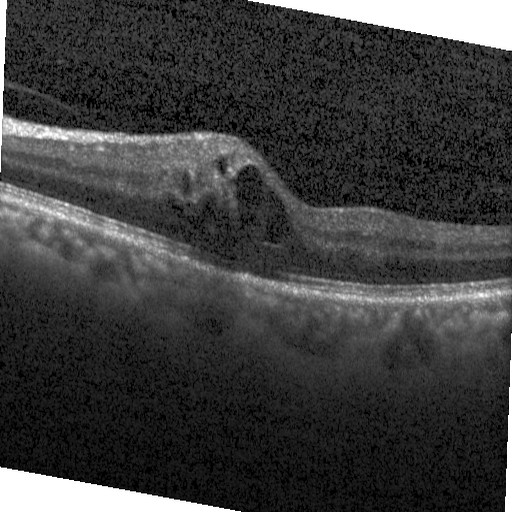 OCT line scan. Horizontal scan through the fovea. Impression: diabetic macular edema (DME).